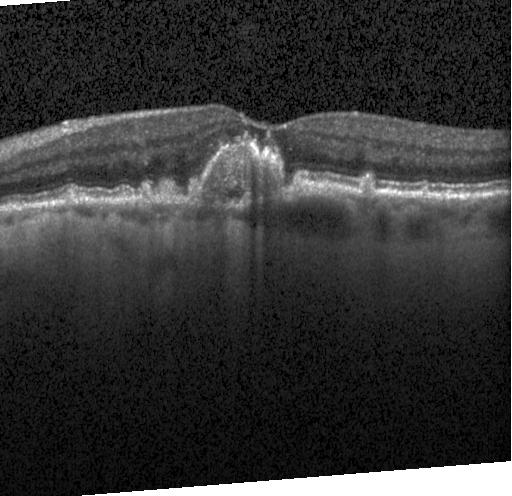

Finding: a choroidal neovascular membrane.